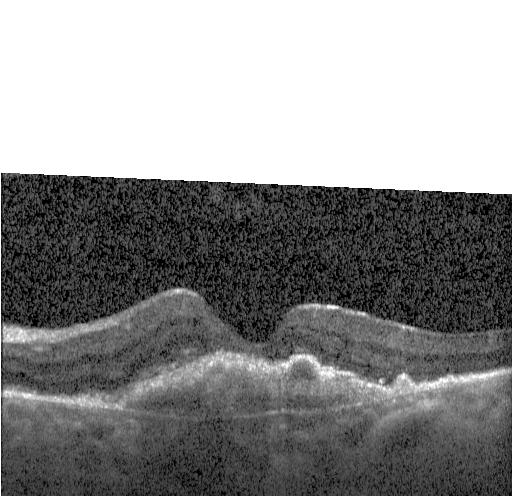 Dx: a choroidal neovascular membrane.